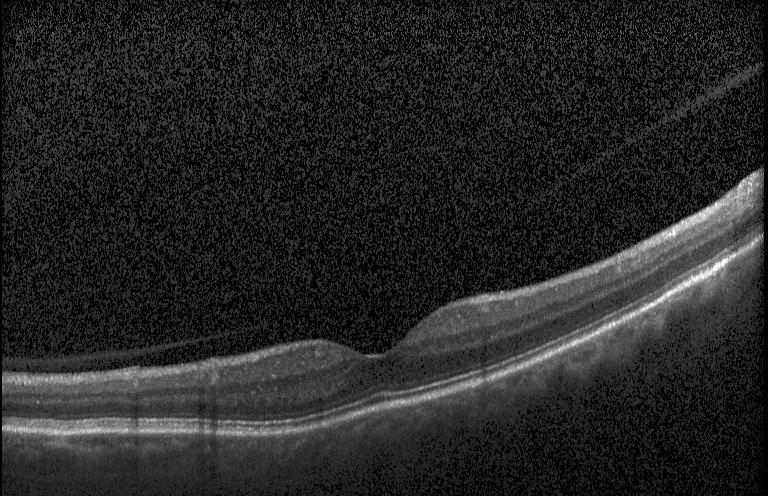

Heidelberg Spectralis. Centered on the fovea. SD-OCT. OCT line scan — No evidence of choroidal neovascularization, diabetic macular edema, or drusen.